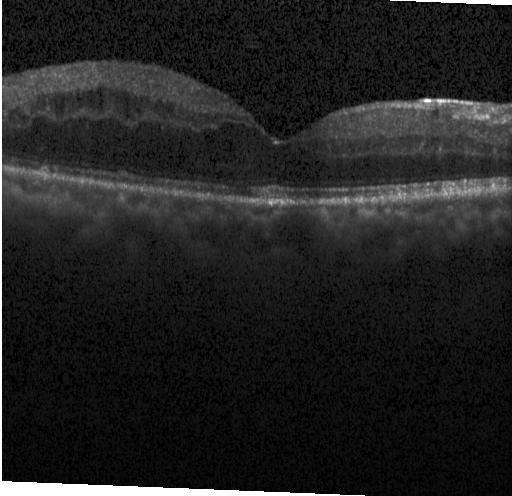 Spectral-domain OCT B-scan: diabetic macular edema (DME).